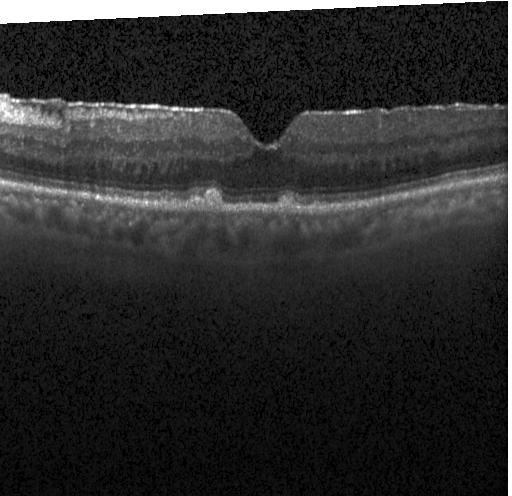
Retinal OCT cross-section — Assessment: multiple drusen.